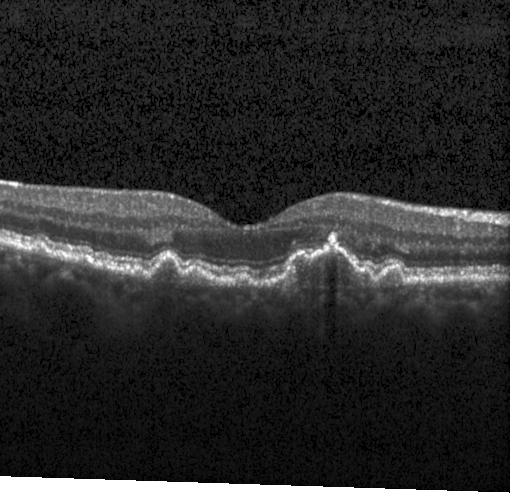 Through the macula, optical coherence tomography B-scan, spectral-domain optical coherence tomography.
Finding: sub-RPE drusenoid deposits.